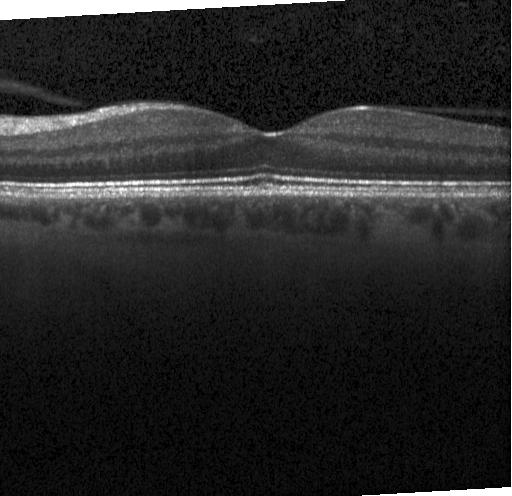

Spectral-domain optical coherence tomography; acquired on a Heidelberg Spectralis; optical coherence tomography B-scan; horizontal scan through the fovea
Diagnosis: no evidence of choroidal neovascularization, diabetic macular edema, or drusen.